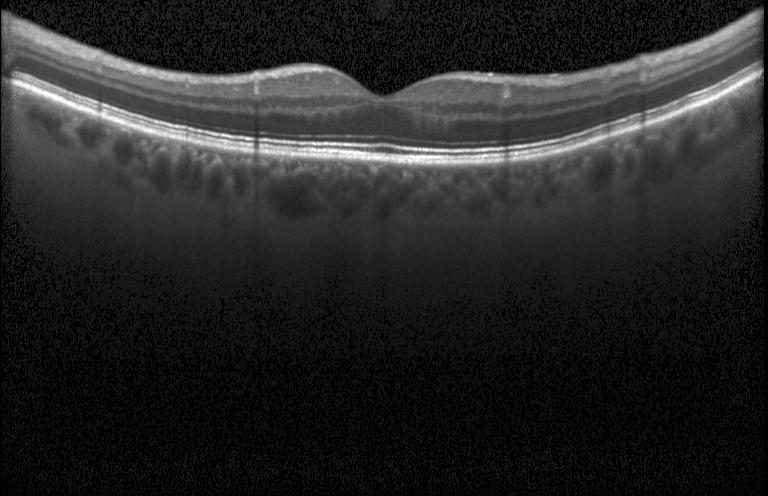

Optical coherence tomography scan.
Dx: no choroidal neovascularization, no diabetic macular edema, and no drusen.